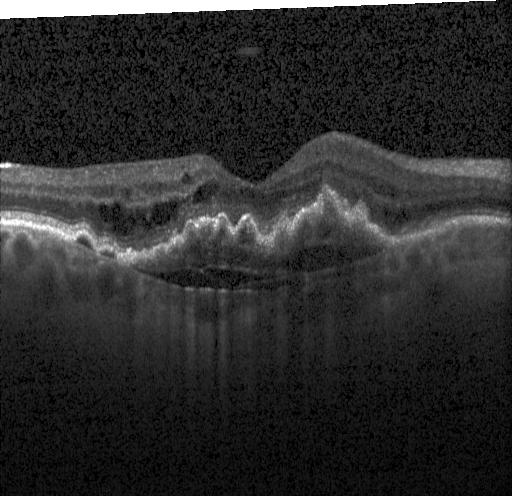

Fovea-centered. SD-OCT. Retinal OCT B-scan.
Choroidal neovascularization (CNV).